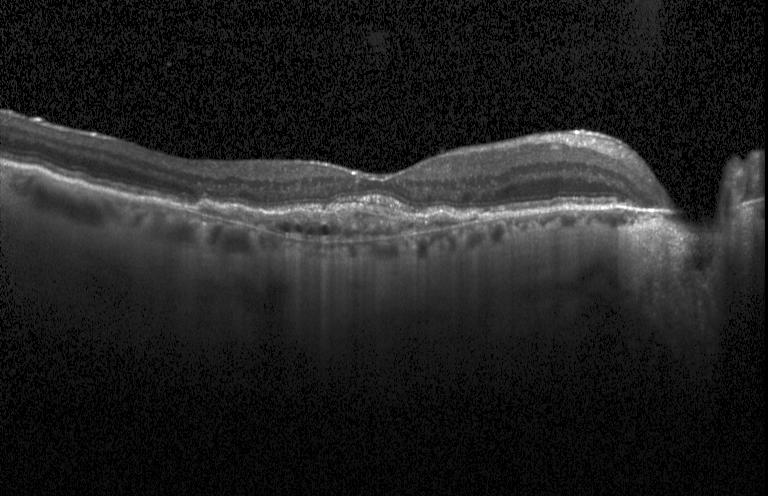

Instrument: Heidelberg Spectralis · optical coherence tomography B-scan. Finding: a choroidal neovascular membrane.